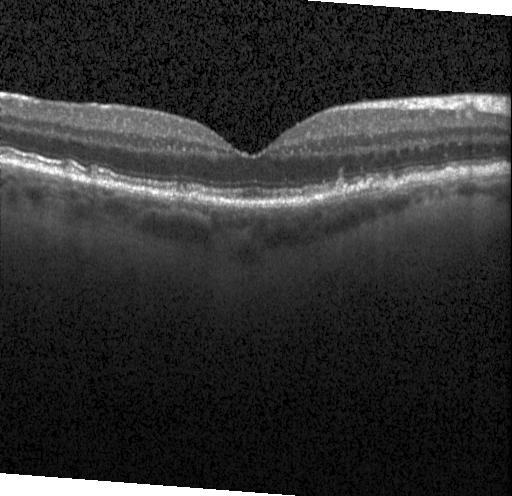
SD-OCT. Heidelberg Spectralis. Retinal OCT cross-section. Finding: multiple drusen.